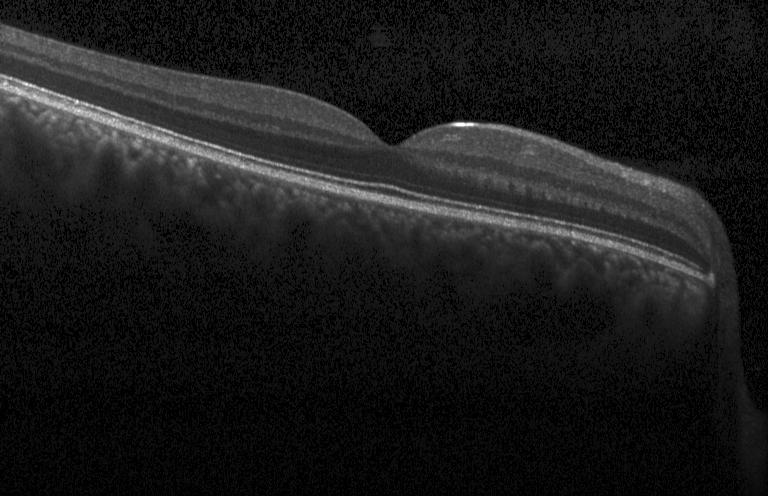

Optical coherence tomography B-scan. SD-OCT. Horizontal scan through the fovea. Heidelberg Spectralis OCT system.
The scan shows no choroidal neovascularization, no diabetic macular edema, and no drusen.